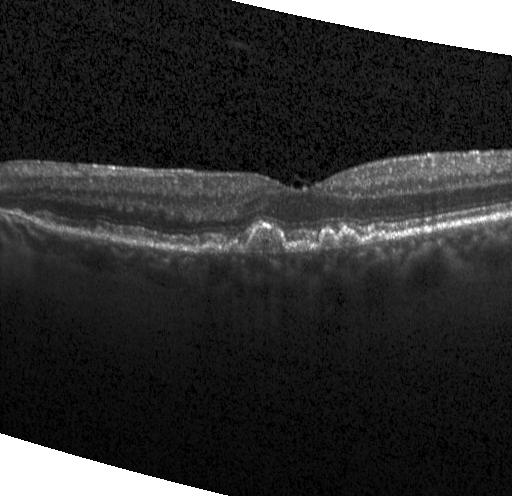 Retinal OCT B-scan, Heidelberg Spectralis, horizontal scan through the fovea, SD-OCT
This B-scan demonstrates multiple drusen.